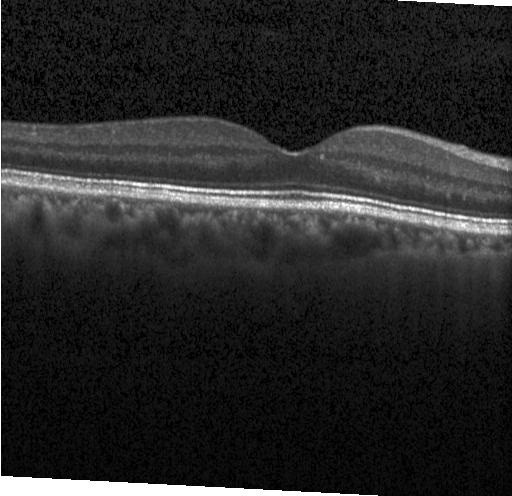 Optical coherence tomography scan — OCT finding: neither CNV, DME, nor drusen.